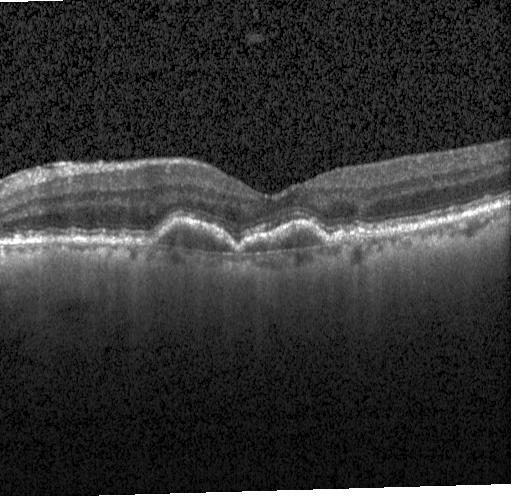 Horizontal scan through the fovea. OCT line scan.
Dx: choroidal neovascularization (CNV).